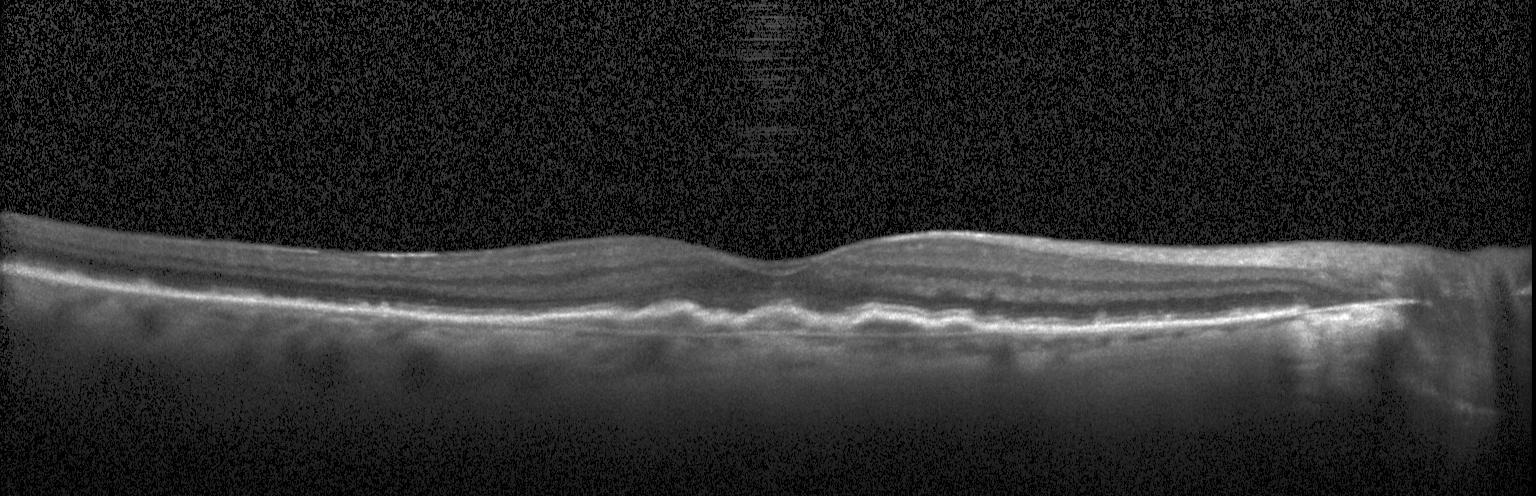

Fovea-centered. Retinal OCT B-scan. Spectral-domain OCT. Acquired on a Heidelberg Spectralis
Assessment: CNV.